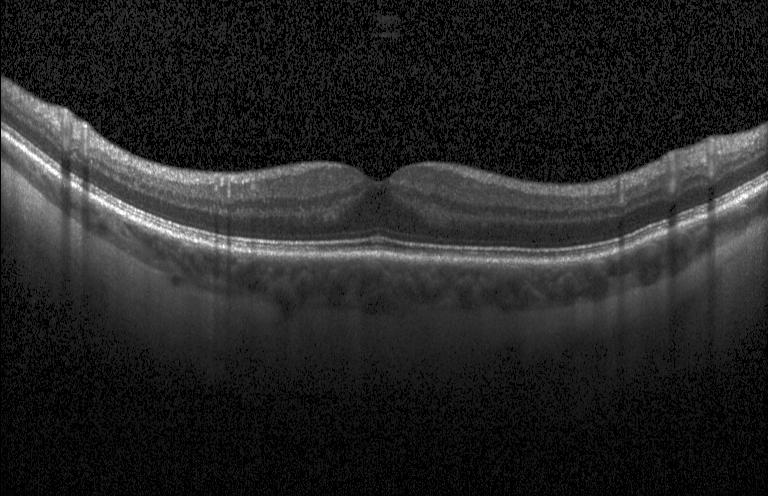
Retinal OCT cross-section
Finding: no choroidal neovascularization, no diabetic macular edema, and no drusen.